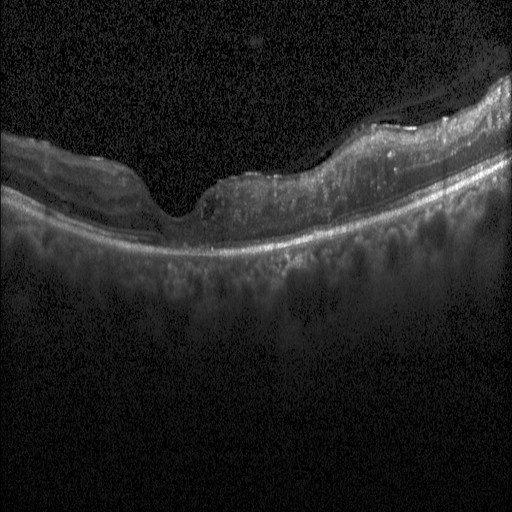 Impression: DME.